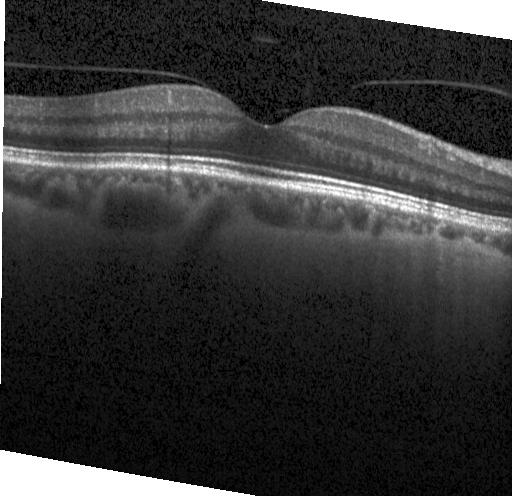

Spectral-domain OCT B-scan: no CNV, DME, or drusen.